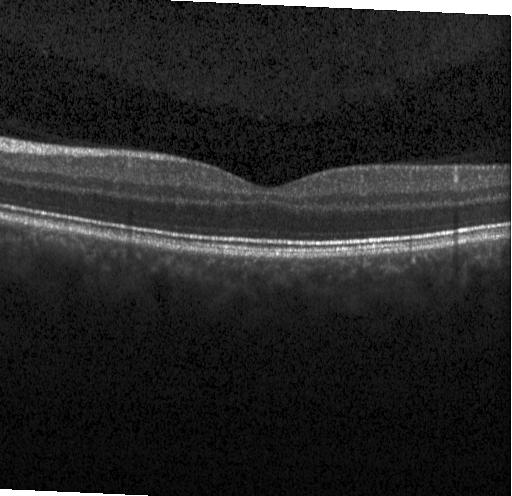 Spectral-domain optical coherence tomography, OCT line scan, Heidelberg Spectralis, fovea-centered
OCT finding: neither CNV, DME, nor drusen.